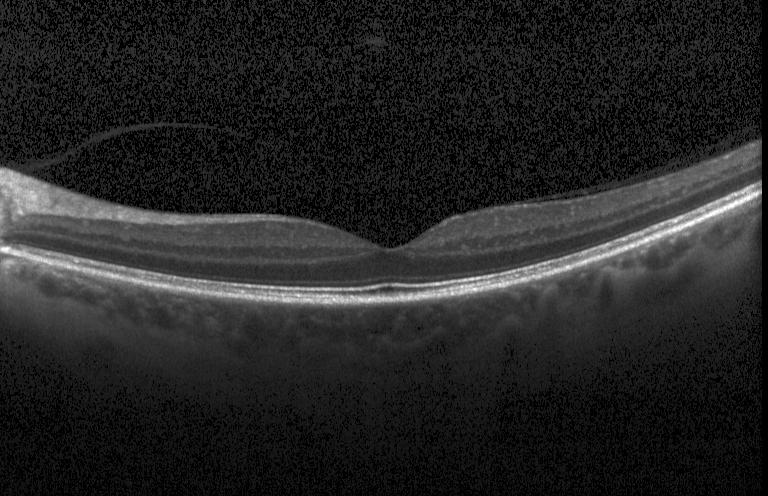

OCT B-scan.
OCT finding: neither CNV, DME, nor drusen.